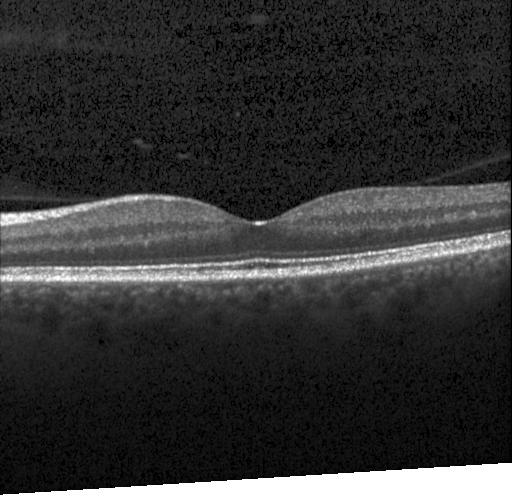 Optical coherence tomography scan — Assessment: no choroidal neovascularization, diabetic macular edema, or drusen.